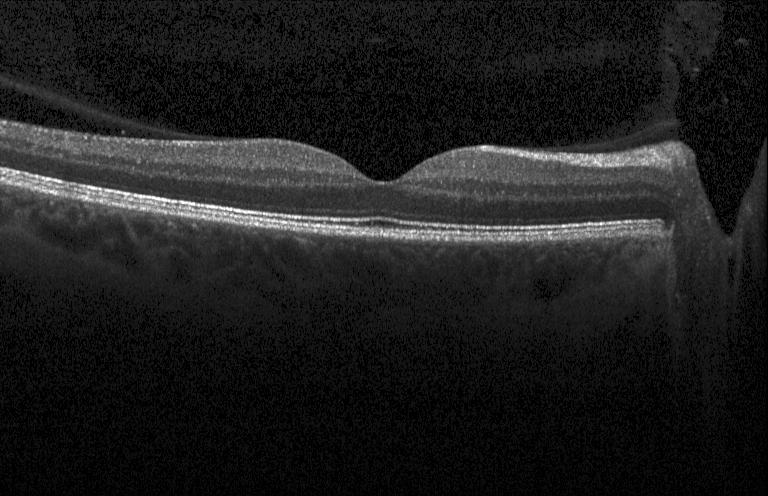
Spectral-domain OCT · retinal OCT cross-section · horizontal scan through the fovea.
This B-scan demonstrates no evidence of CNV, DME, or drusen.